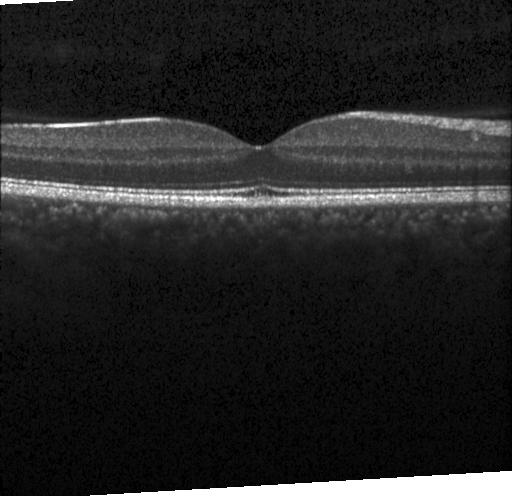

OCT scan showing no choroidal neovascularization, no diabetic macular edema, and no drusen.